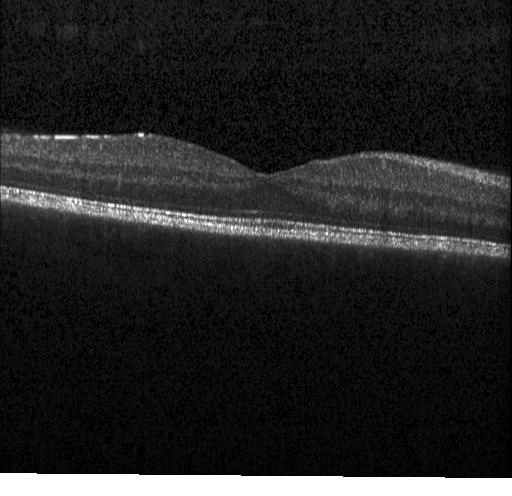

Heidelberg Spectralis OCT system · OCT line scan · SD-OCT — Diagnosis: no evidence of choroidal neovascularization, diabetic macular edema, or drusen.